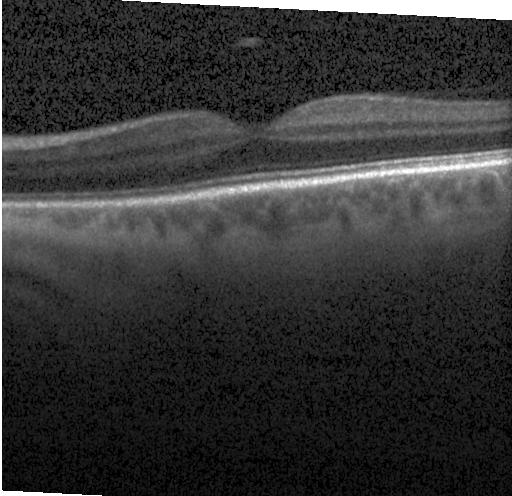

Finding: no choroidal neovascularization, diabetic macular edema, or drusen.